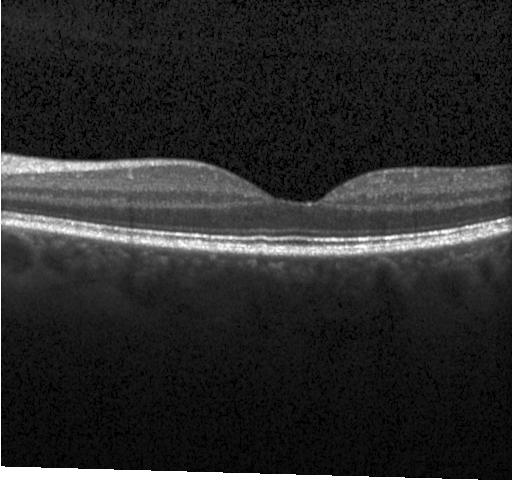
Retinal OCT cross-section, spectral-domain OCT.
Diagnosis: no evidence of choroidal neovascularization, diabetic macular edema, or drusen.